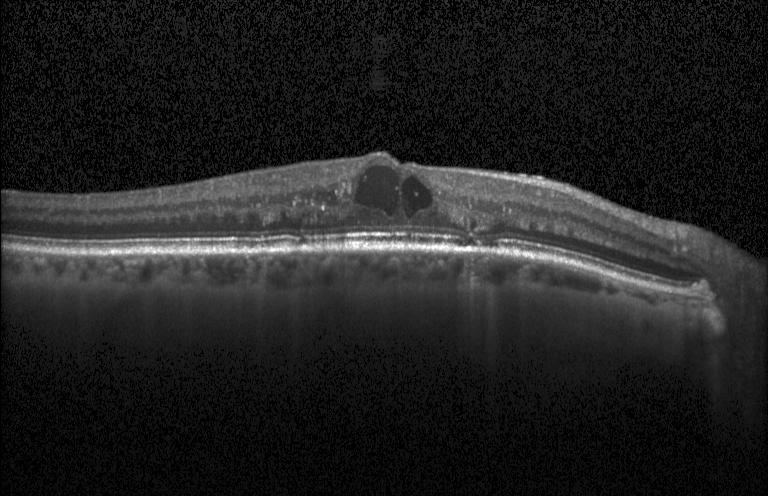

Impression: diabetic macular edema (DME).